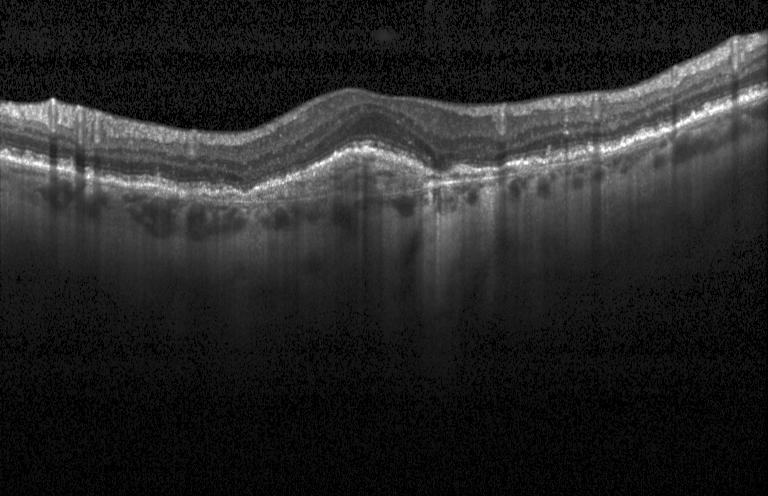
Spectral-domain optical coherence tomography, retinal OCT cross-section, instrument: Heidelberg Spectralis — A choroidal neovascular membrane.